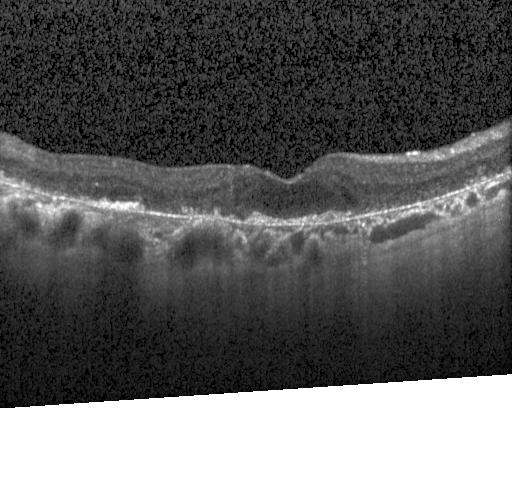 Heidelberg Spectralis OCT system; fovea-centered; SD-OCT; optical coherence tomography B-scan — Impression: choroidal neovascularization (CNV).